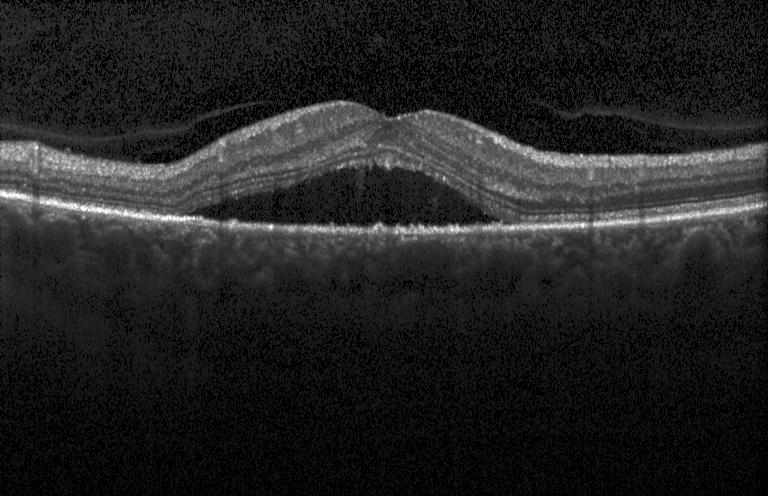
Optical coherence tomography scan, through the macula — The scan shows choroidal neovascularization.